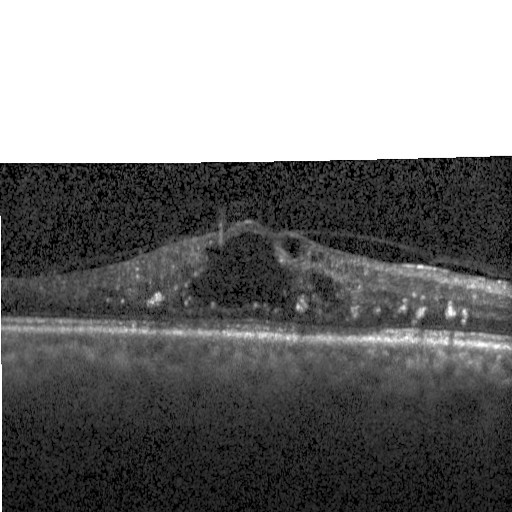
OCT B-scan showing DME.